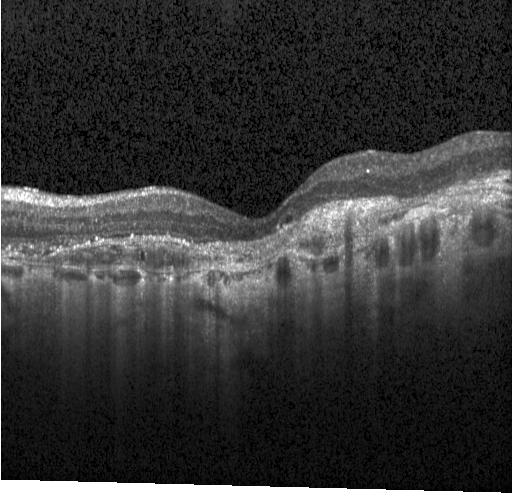
Optical coherence tomography scan — Diagnosis: choroidal neovascularization.